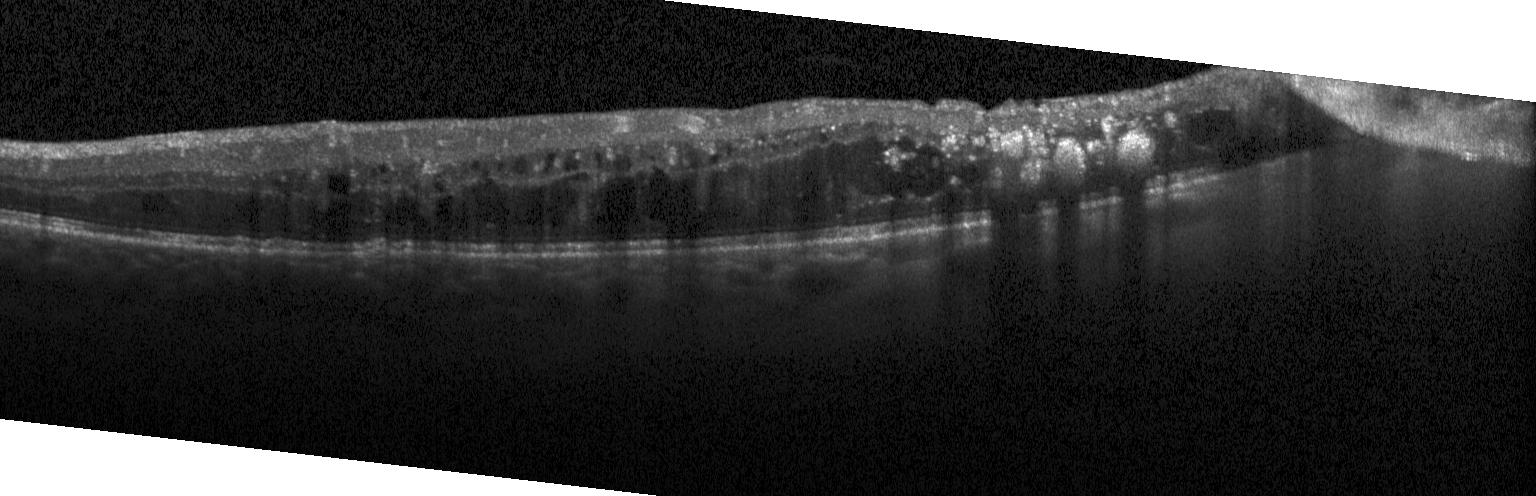

OCT line scan
Diagnosis: DME.